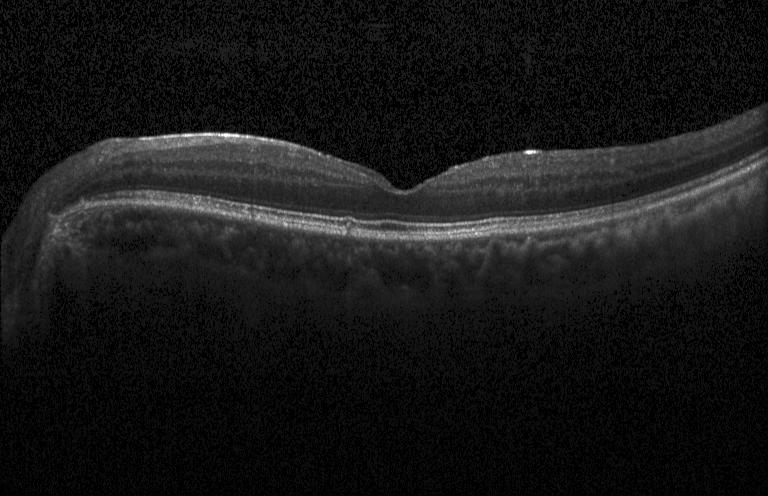
Finding: no CNV, DME, or drusen.